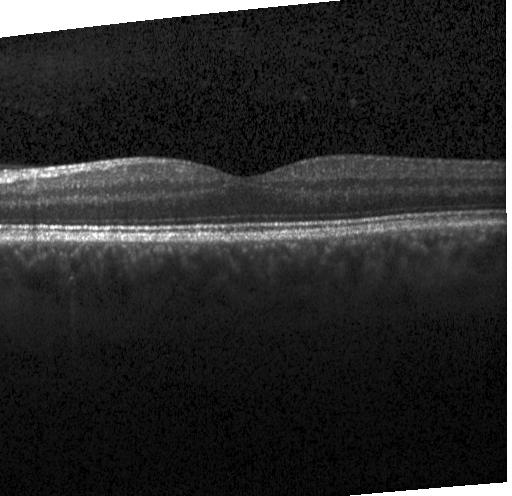 Spectral-domain optical coherence tomography, retinal OCT cross-section. Finding: neither choroidal neovascularization, diabetic macular edema, nor drusen.